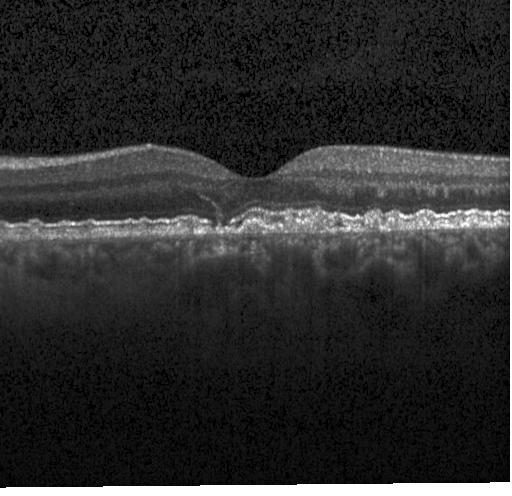 Macular OCT: multiple drusen.